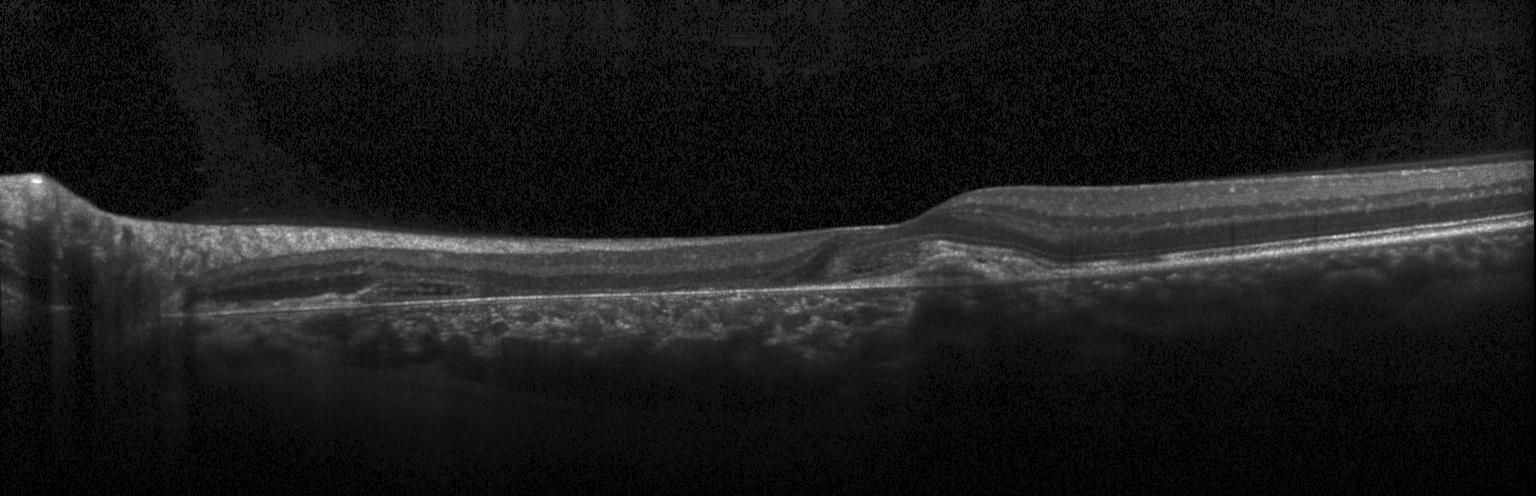
Heidelberg Spectralis OCT system; OCT B-scan; spectral-domain OCT. The scan shows choroidal neovascularization.